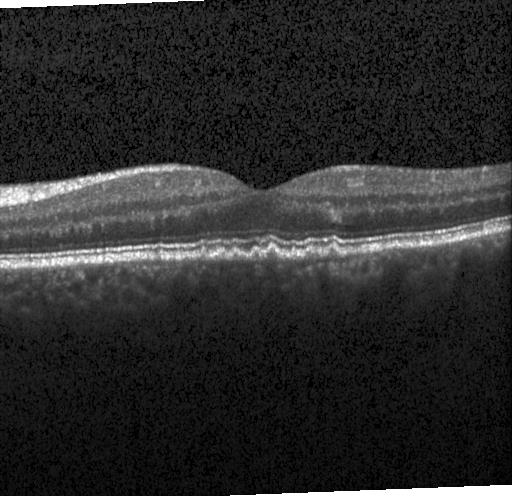 Assessment: multiple drusen.